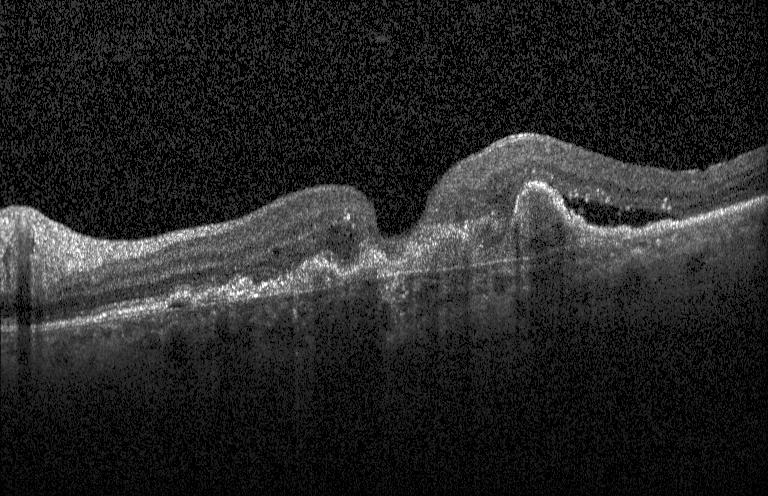

Spectral-domain optical coherence tomography. Heidelberg Spectralis OCT system. Macular scan. Retinal OCT cross-section. Finding: choroidal neovascularization (CNV).